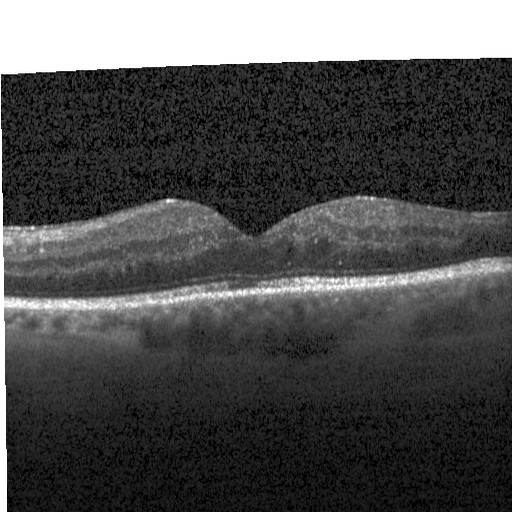 Retinal OCT B-scan; centered on the fovea. Diagnosis: diabetic macular edema.